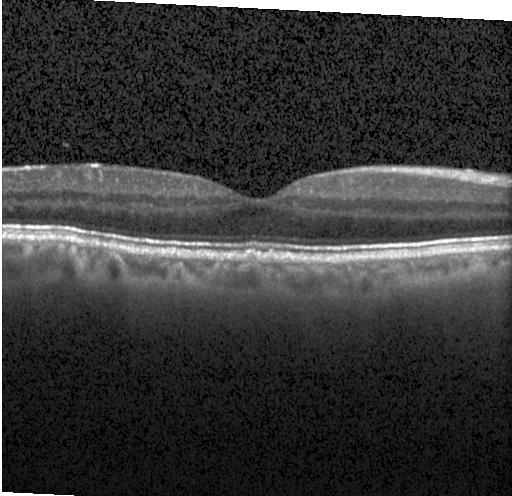 Finding: neither CNV, DME, nor drusen.